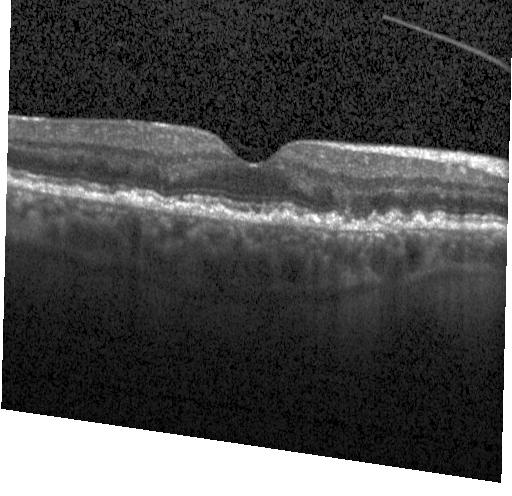

The scan shows multiple drusen.